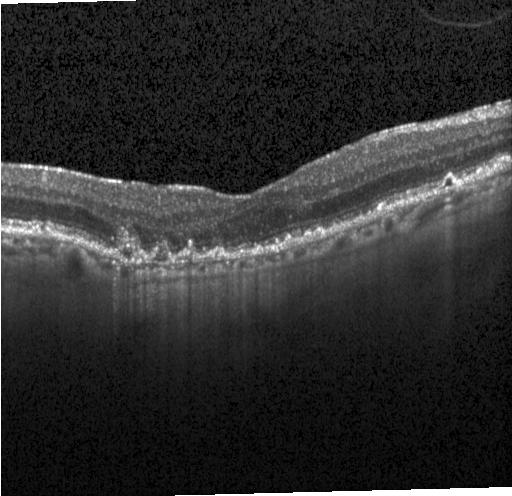

OCT line scan; spectral-domain optical coherence tomography.
Impression: a choroidal neovascular membrane.